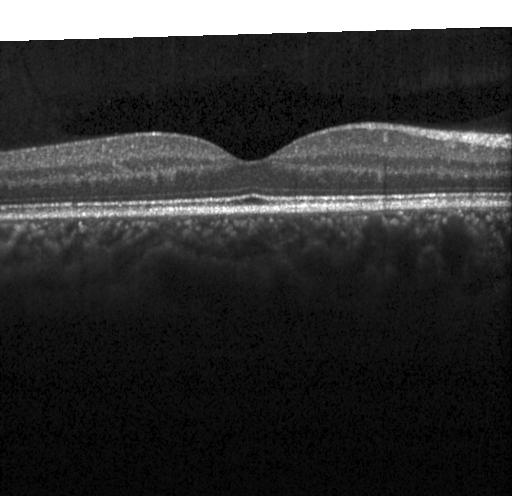
Assessment: no CNV, DME, or drusen.